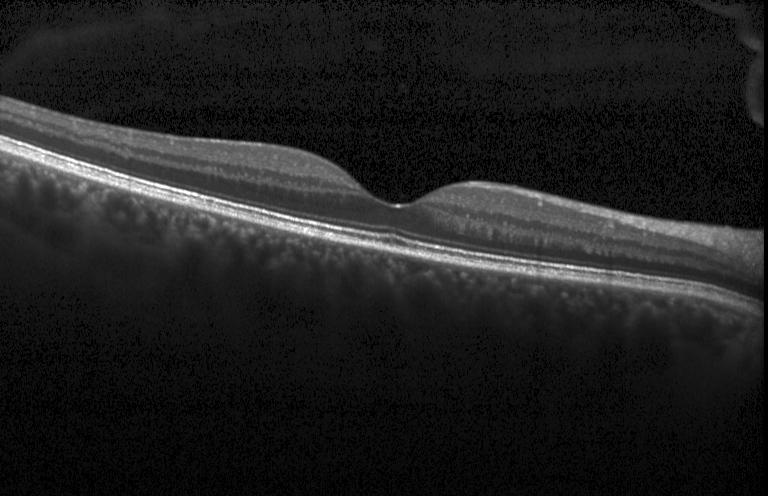
Optical coherence tomography scan — Impression: no CNV, no DME, and no drusen.